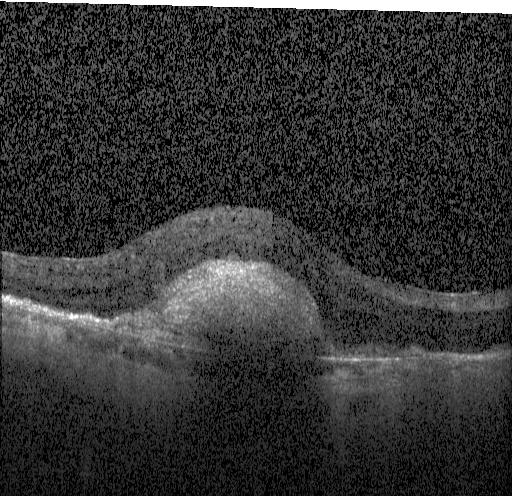

Diagnosis: a choroidal neovascular membrane.